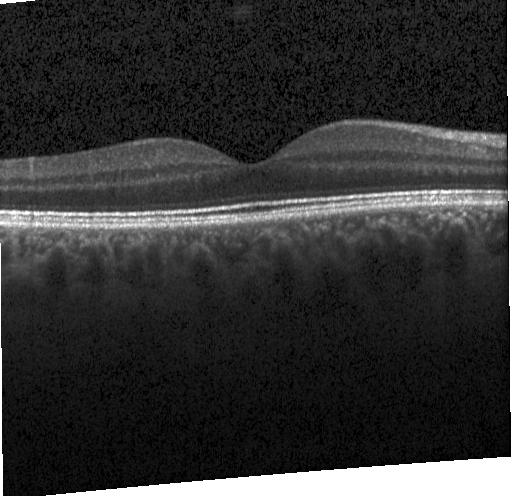
Heidelberg Spectralis OCT system; optical coherence tomography B-scan
Impression: no choroidal neovascularization, no diabetic macular edema, and no drusen.